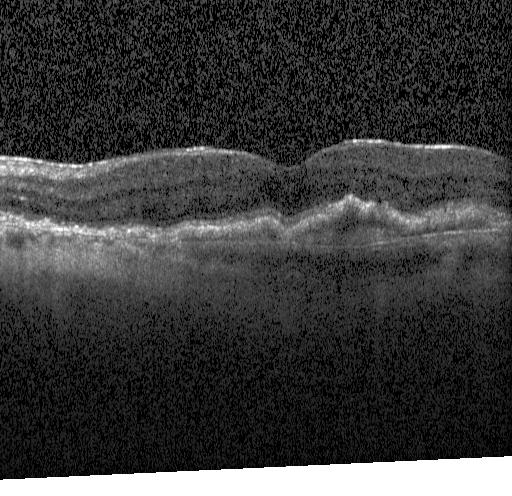
Optical coherence tomography scan
The scan shows a choroidal neovascular membrane.